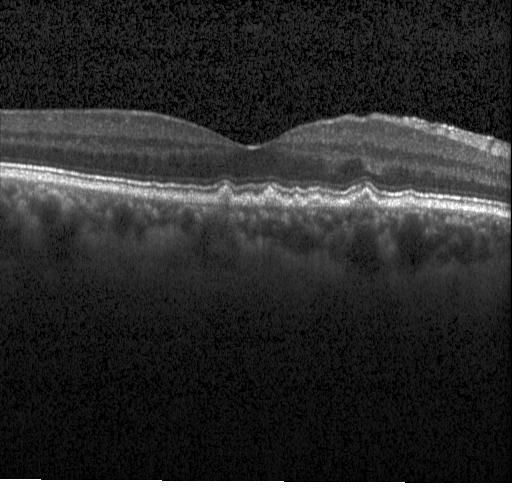 OCT scan showing sub-RPE drusenoid deposits.